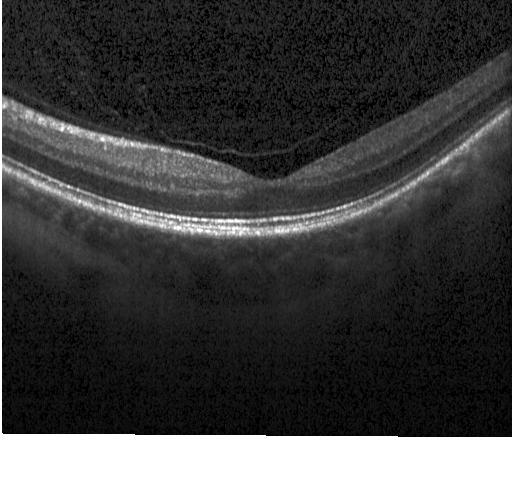

OCT line scan; horizontal scan through the fovea.
No evidence of choroidal neovascularization, diabetic macular edema, or drusen.